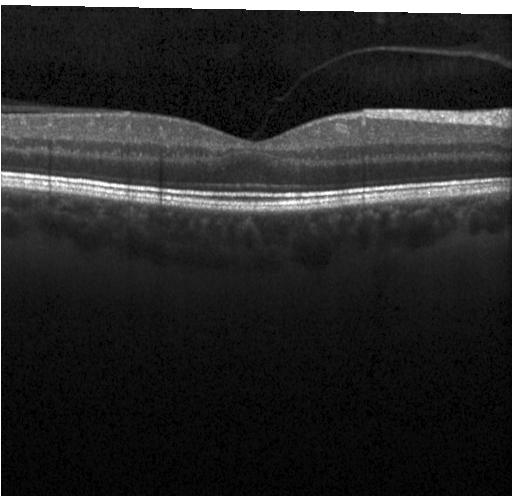 Retinal OCT B-scan
Dx: no choroidal neovascularization, diabetic macular edema, or drusen.